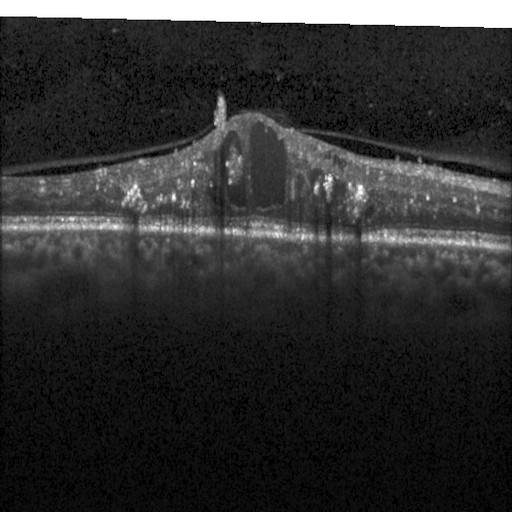
Retinal OCT B-scan, SD-OCT, macular scan, instrument: Heidelberg Spectralis — Macular OCT: DME.